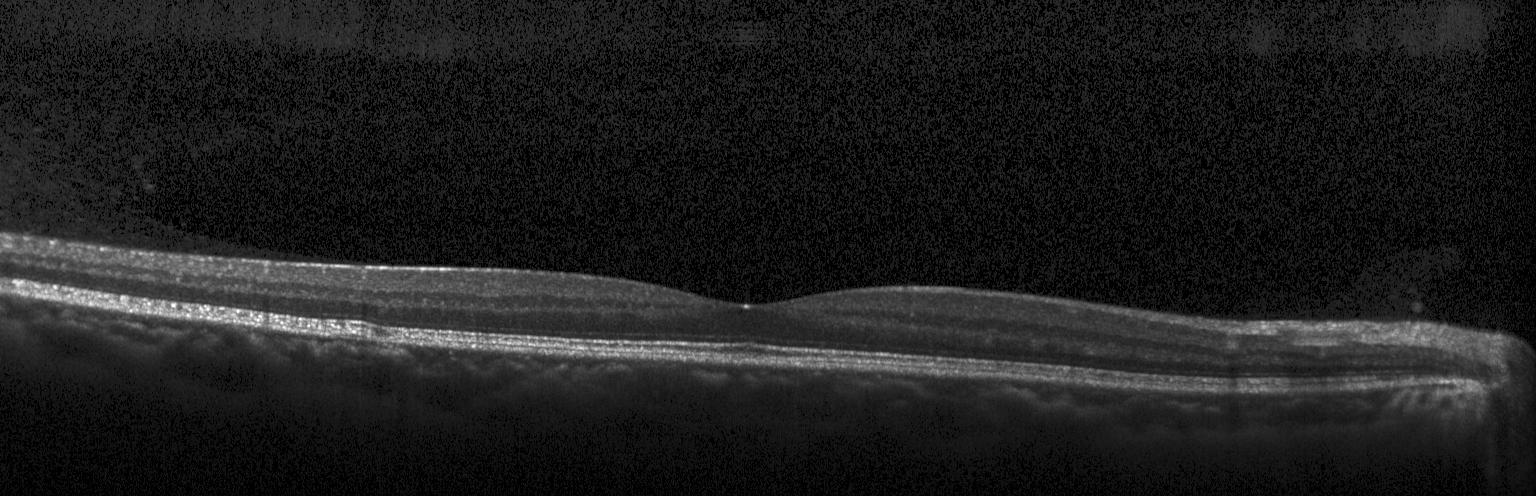 Retinal OCT cross-section. OCT finding: no choroidal neovascularization, diabetic macular edema, or drusen.